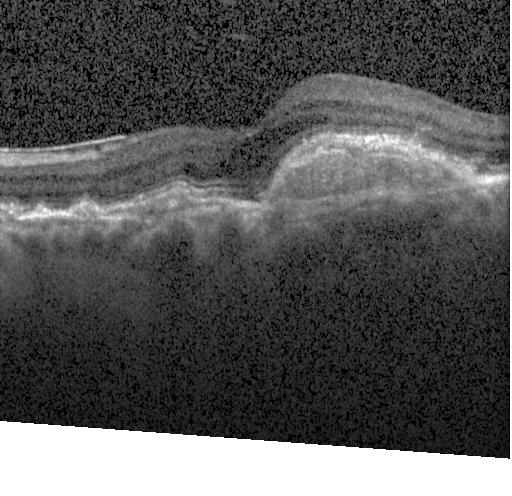
Retinal OCT B-scan, spectral-domain OCT.
Diagnosis: a choroidal neovascular membrane.